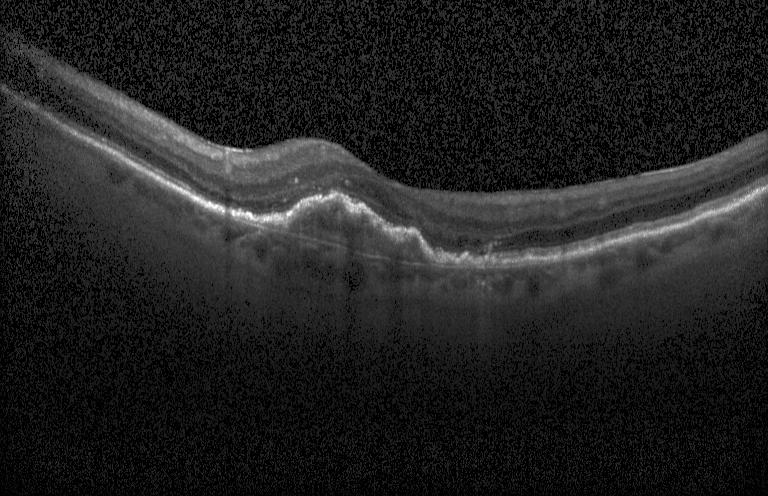 OCT finding: a choroidal neovascular membrane.